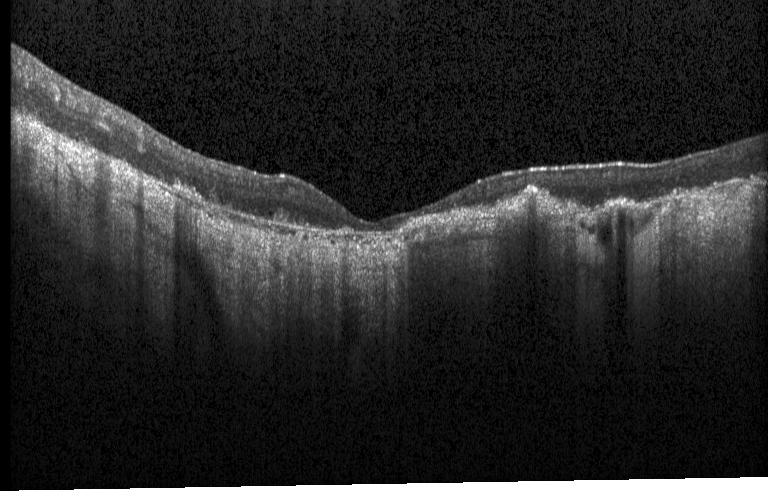

Spectral-domain OCT B-scan: a choroidal neovascular membrane.